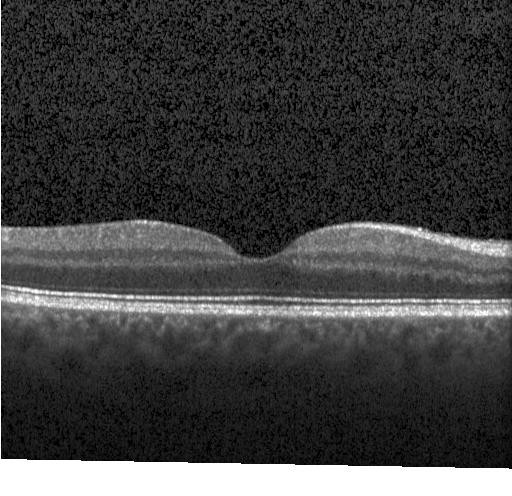
SD-OCT · Heidelberg Spectralis · OCT B-scan · through the macula — Neither choroidal neovascularization, diabetic macular edema, nor drusen.